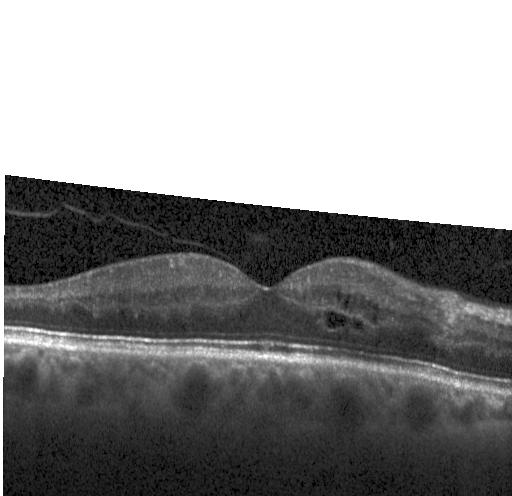
Heidelberg Spectralis · through the macula · spectral-domain OCT · OCT line scan. OCT finding: DME.